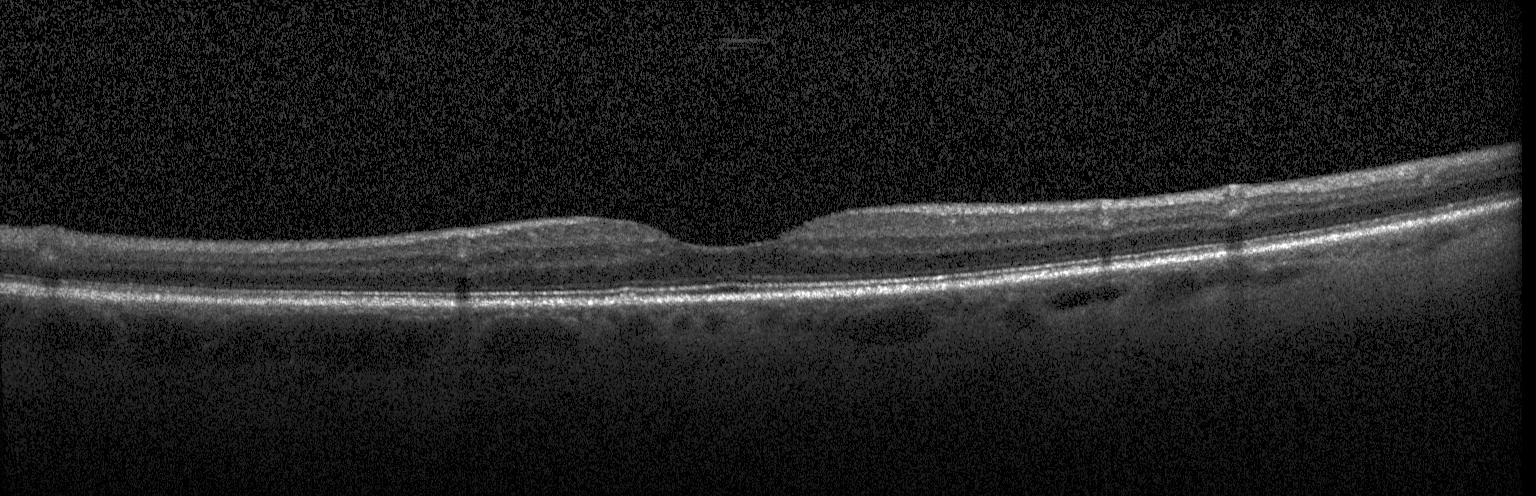
OCT finding: neither choroidal neovascularization, diabetic macular edema, nor drusen.